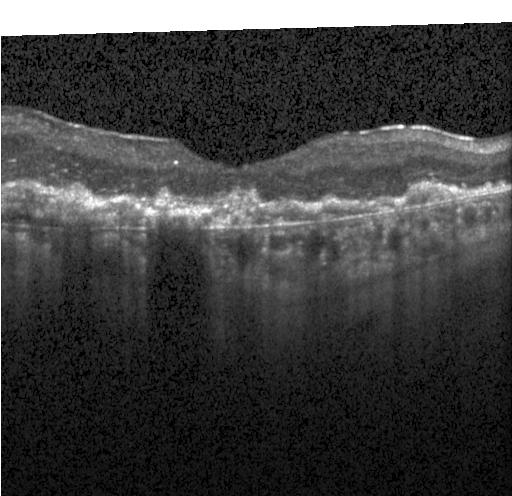

SD-OCT; OCT line scan; fovea-centered; Heidelberg Spectralis
Finding: CNV.